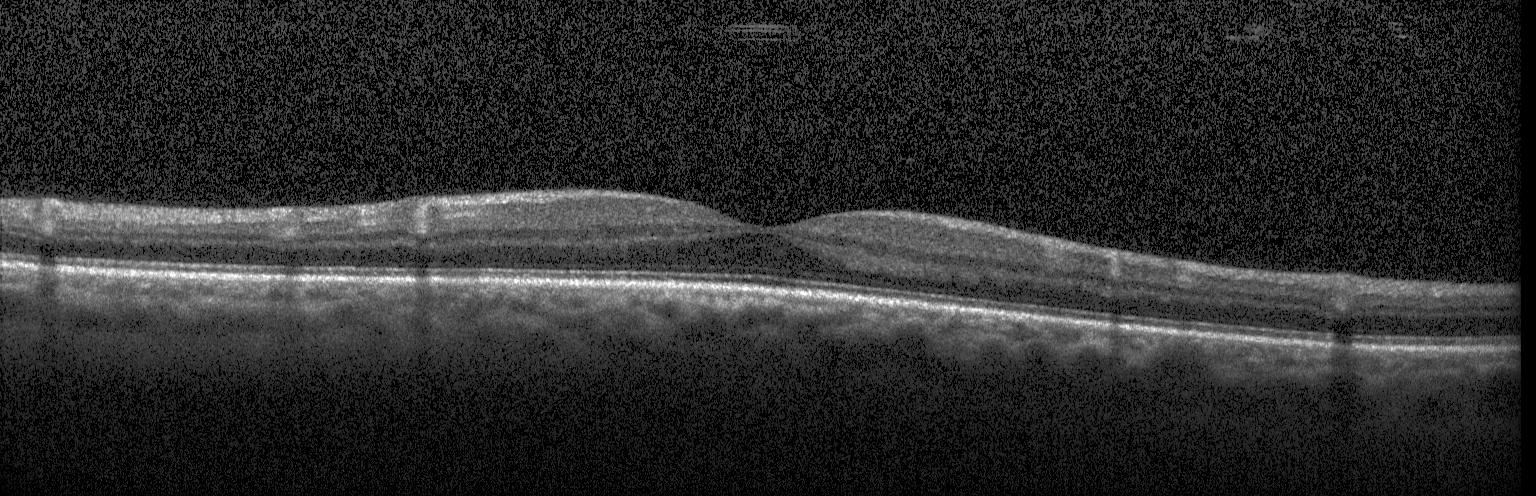
Heidelberg Spectralis OCT system, optical coherence tomography B-scan, through the macula
Finding: no evidence of choroidal neovascularization, diabetic macular edema, or drusen.